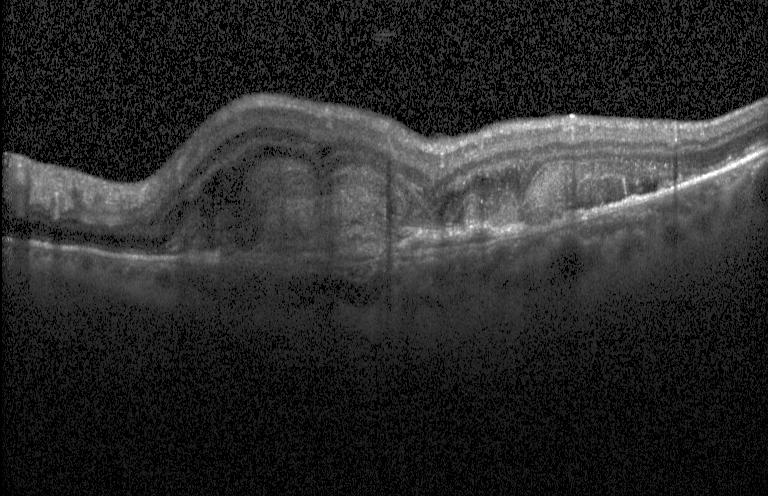
SD-OCT · retinal OCT B-scan · macular scan · Heidelberg Spectralis — Choroidal neovascularization (CNV).